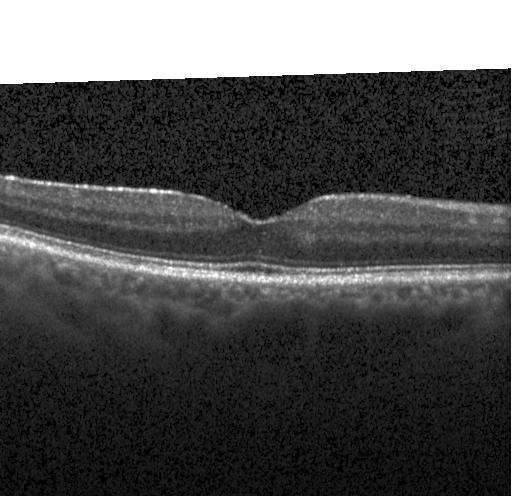 Retinal OCT cross-section. Assessment: neither CNV, DME, nor drusen.